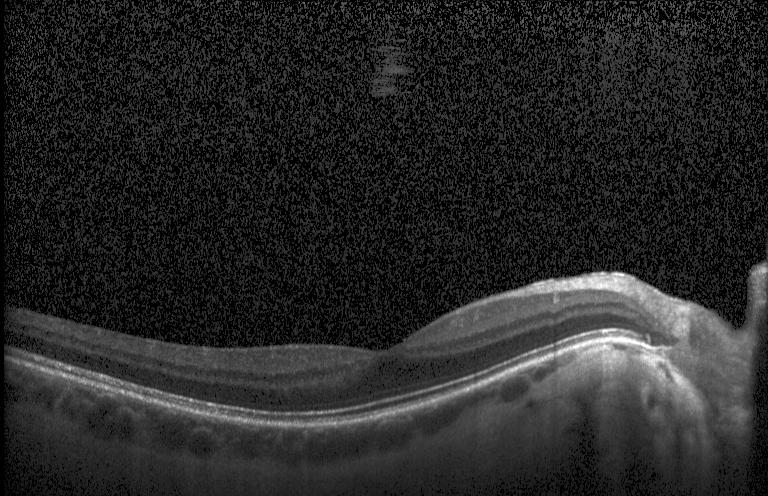 Retinal OCT cross-section showing no choroidal neovascularization, no diabetic macular edema, and no drusen.